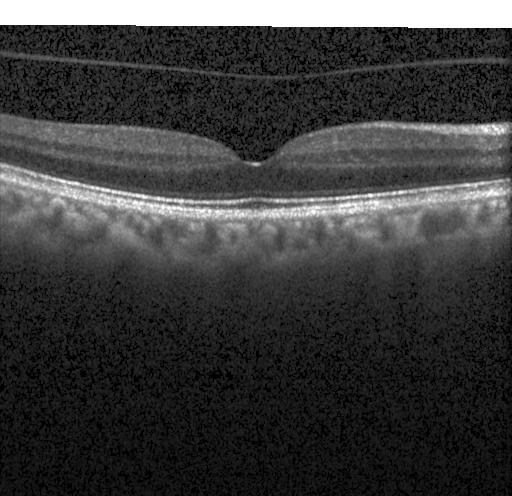
Optical coherence tomography scan · SD-OCT
Finding: neither choroidal neovascularization, diabetic macular edema, nor drusen.